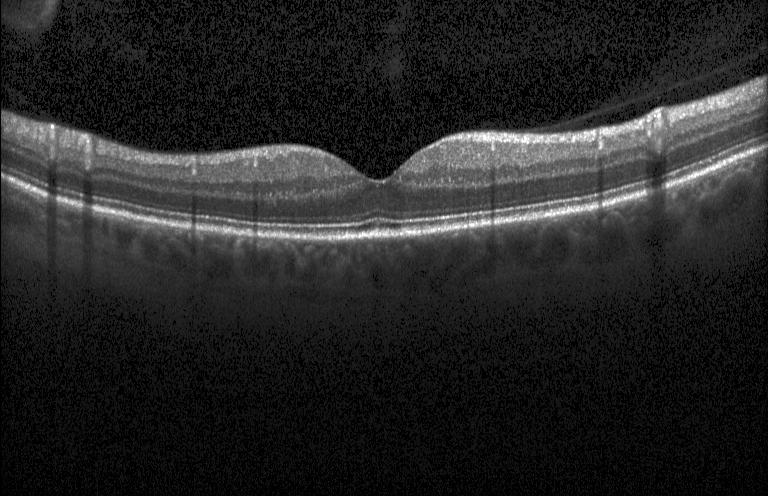

Heidelberg Spectralis OCT system · fovea-centered · retinal OCT cross-section · SD-OCT. Assessment: neither choroidal neovascularization, diabetic macular edema, nor drusen.